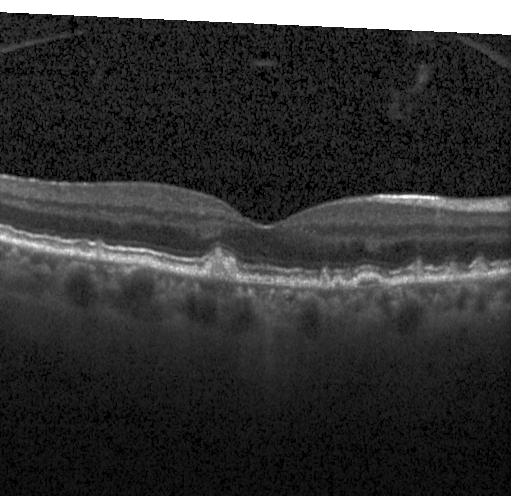
Retinal OCT cross-section showing drusen.